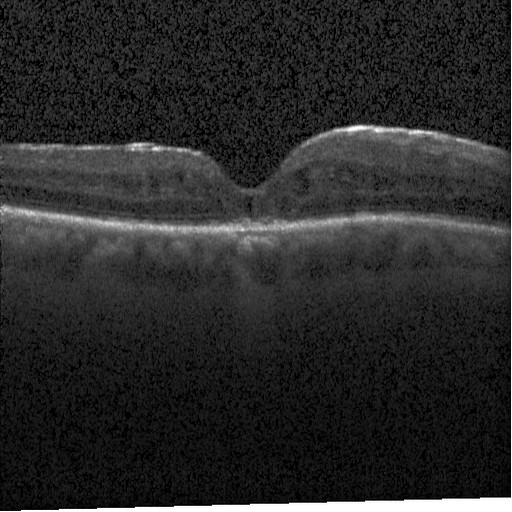

Diagnosis: DME.